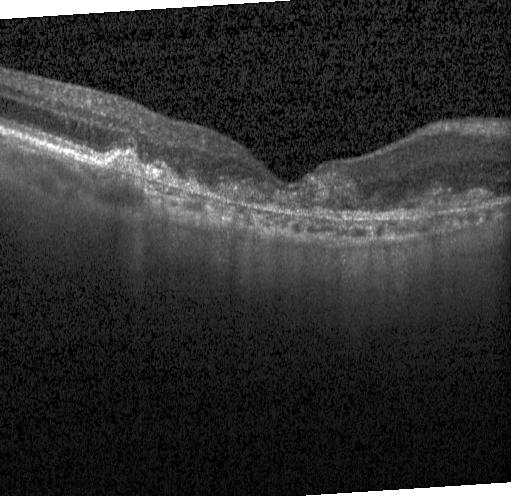

Retinal OCT cross-section. Instrument: Heidelberg Spectralis.
Dx: a choroidal neovascular membrane.